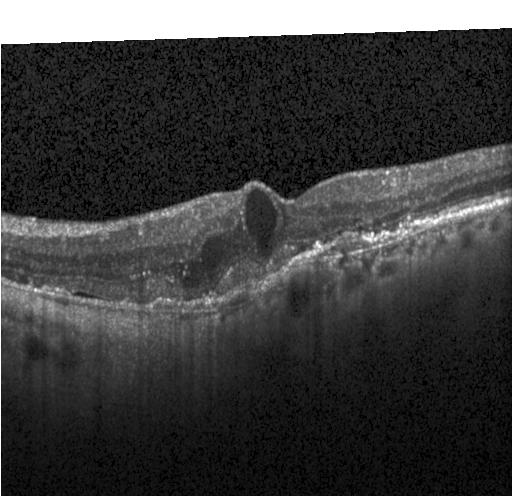
Acquired on a Heidelberg Spectralis · OCT B-scan · fovea-centered · spectral-domain optical coherence tomography — Macular OCT: choroidal neovascularization.